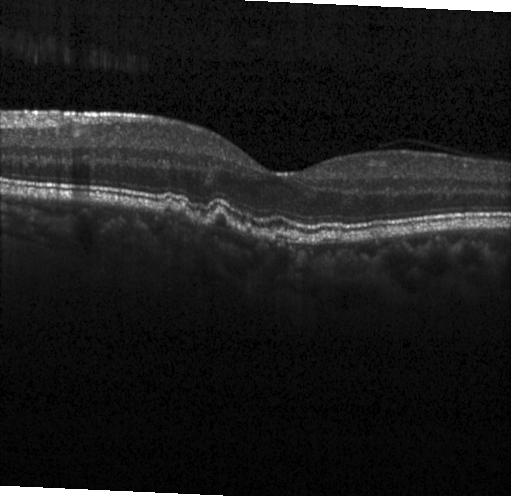
This B-scan demonstrates drusen.